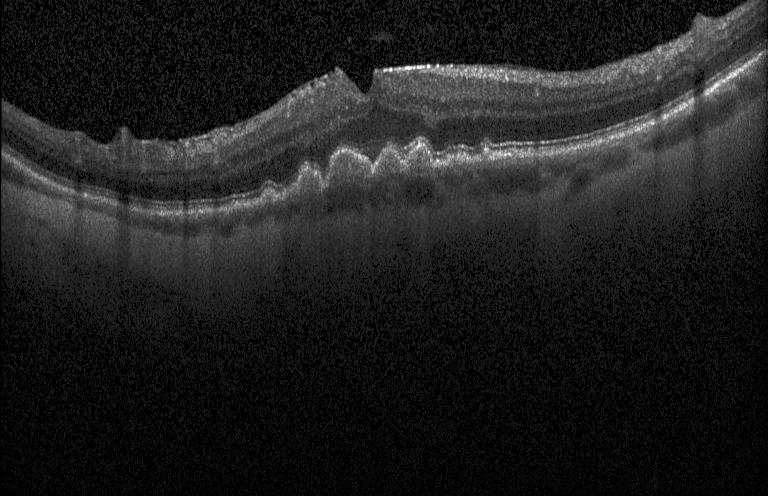

Heidelberg Spectralis; OCT B-scan. Macular OCT: multiple drusen.